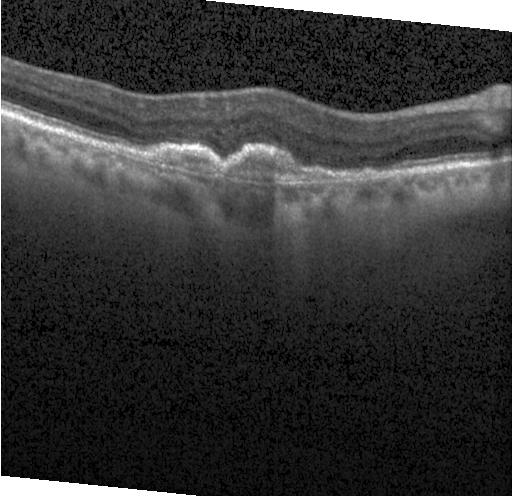 OCT finding: a choroidal neovascular membrane.